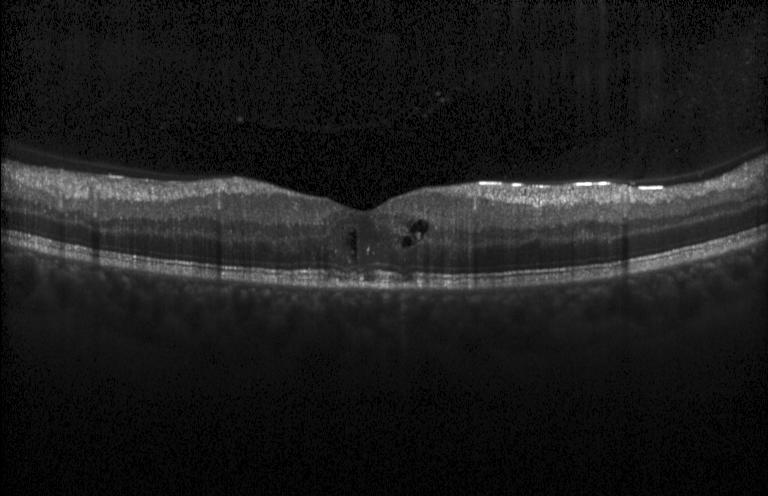
Acquired on a Heidelberg Spectralis · optical coherence tomography B-scan · spectral-domain optical coherence tomography · centered on the fovea
This B-scan demonstrates diabetic macular edema (DME).